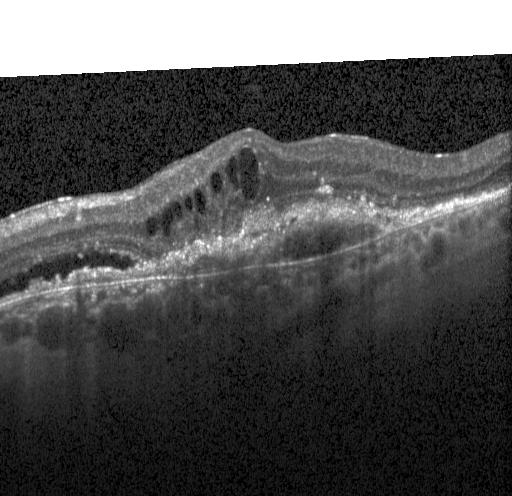
OCT line scan.
Assessment: choroidal neovascularization.